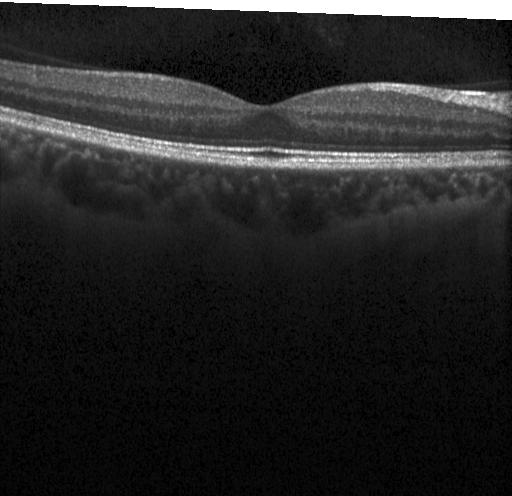

Neither CNV, DME, nor drusen.